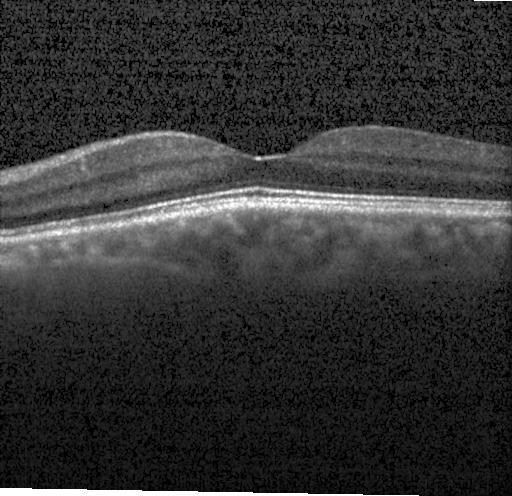
Spectral-domain optical coherence tomography · horizontal scan through the fovea · optical coherence tomography B-scan · Heidelberg Spectralis OCT system
Assessment: neither choroidal neovascularization, diabetic macular edema, nor drusen.